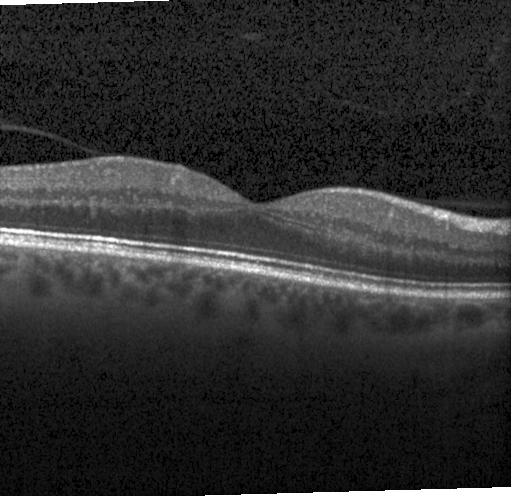 Through the macula. Optical coherence tomography scan. Spectral-domain optical coherence tomography — Diagnosis: no CNV, DME, or drusen.